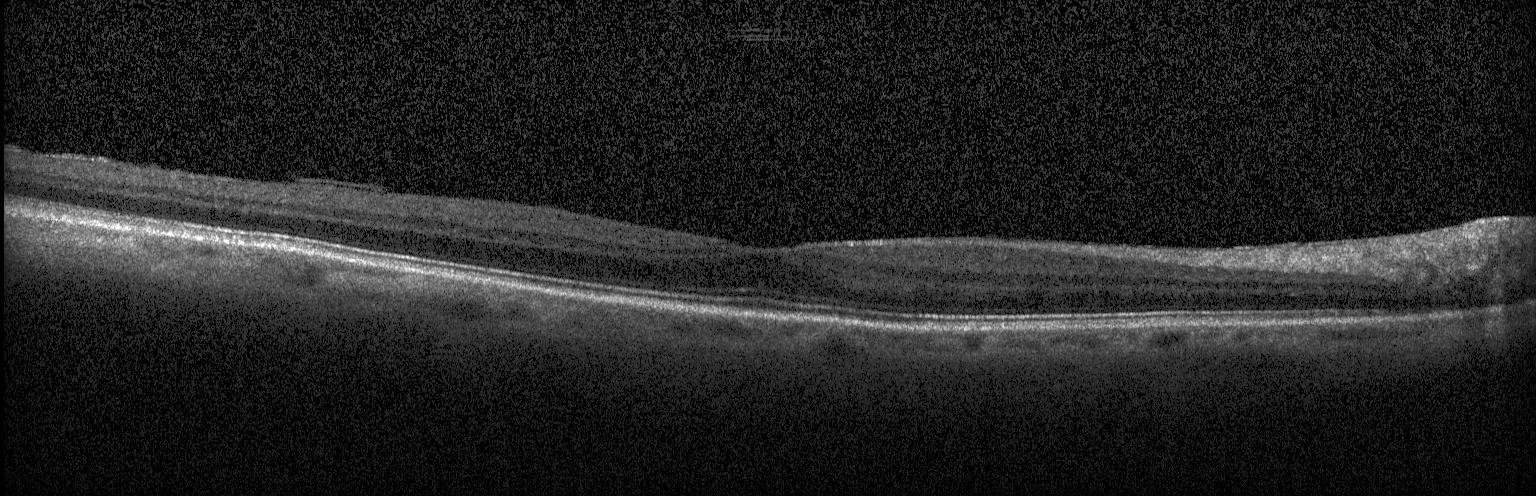

Dx: no choroidal neovascularization, no diabetic macular edema, and no drusen.